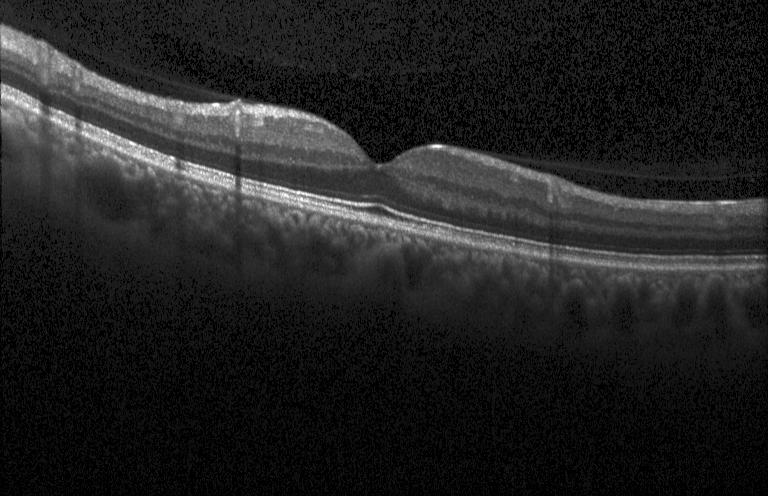 Optical coherence tomography scan
Impression: neither choroidal neovascularization, diabetic macular edema, nor drusen.